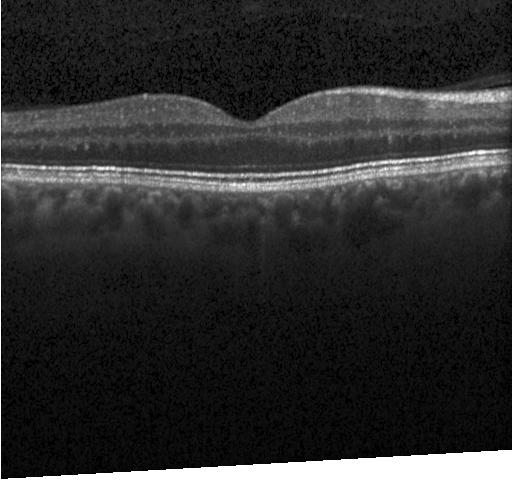
OCT scan showing neither CNV, DME, nor drusen.